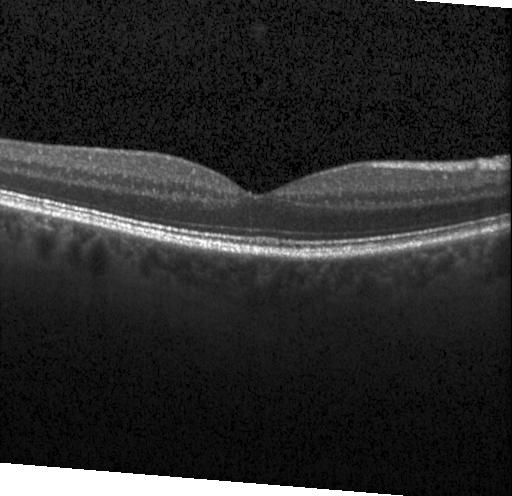
OCT finding: no evidence of CNV, DME, or drusen.